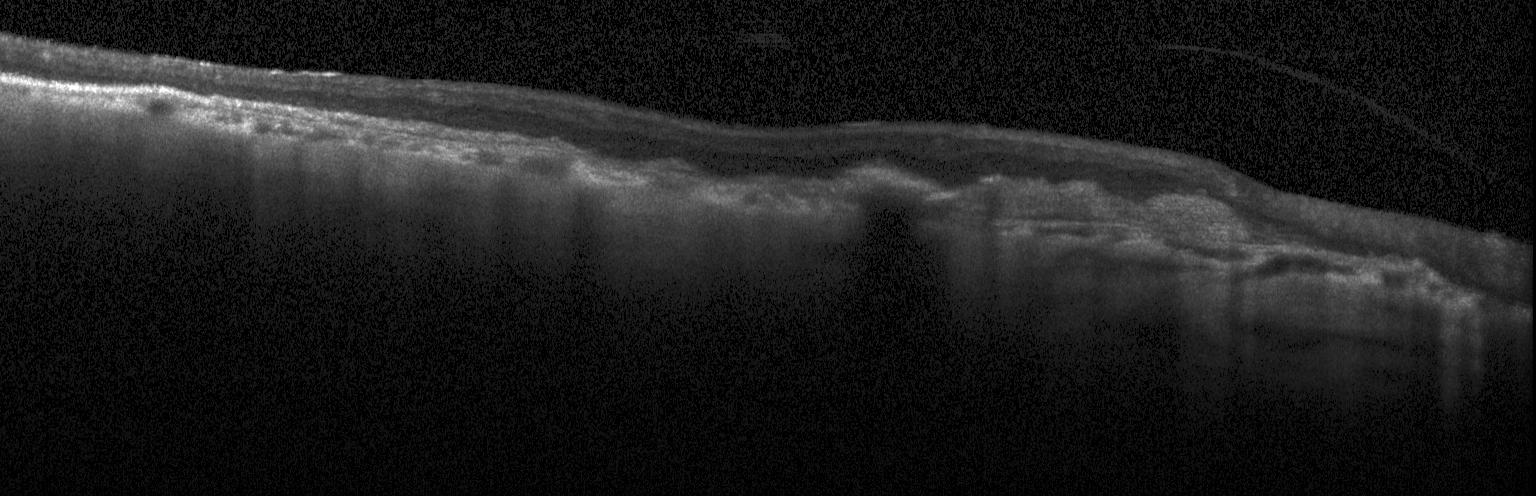
Optical coherence tomography scan. Dx: a choroidal neovascular membrane.